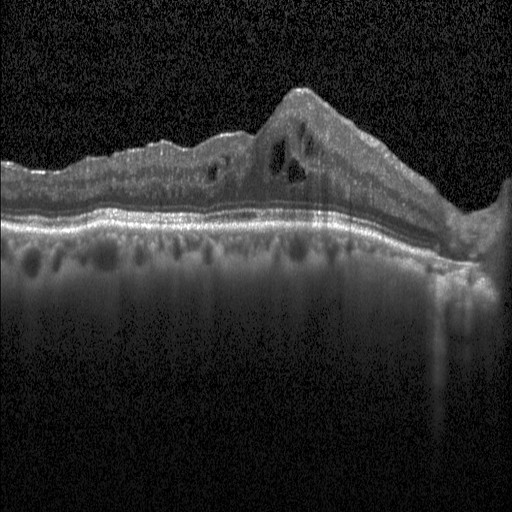
OCT B-scan, SD-OCT, instrument: Heidelberg Spectralis
This B-scan demonstrates diabetic macular edema (DME).